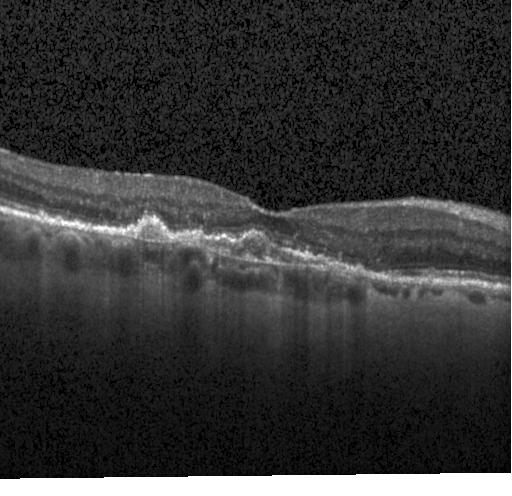

Finding: a choroidal neovascular membrane.